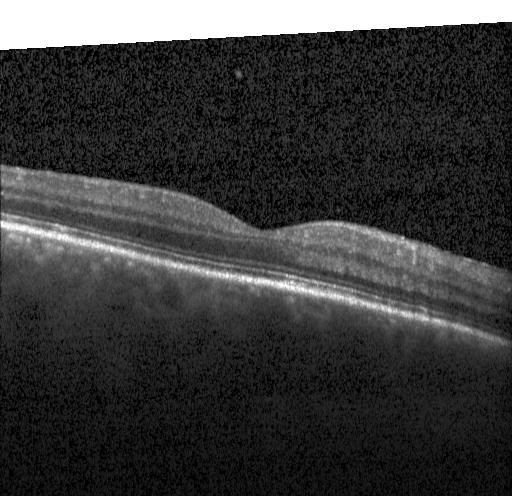
No choroidal neovascularization, diabetic macular edema, or drusen.